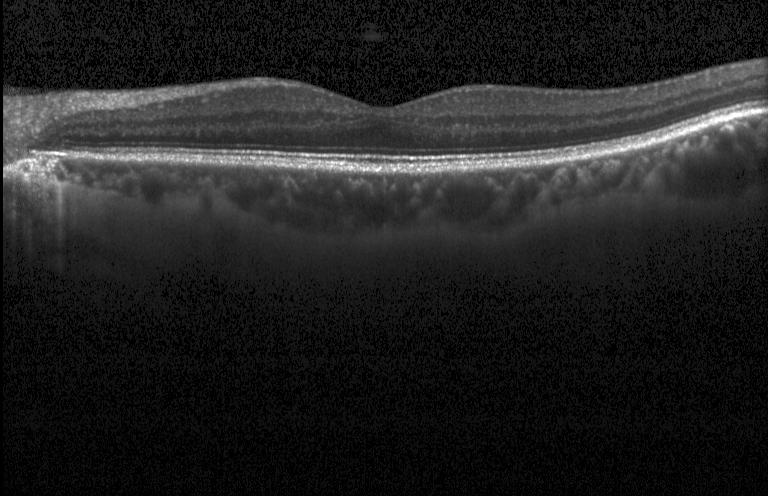

OCT line scan.
This B-scan demonstrates no evidence of CNV, DME, or drusen.